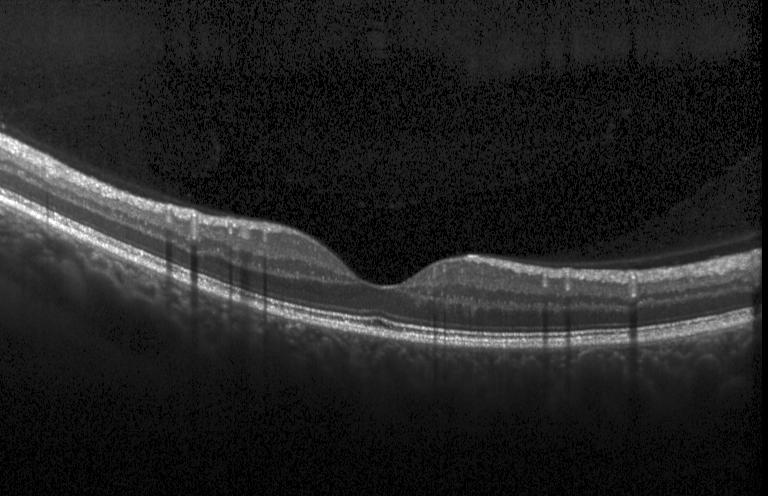
The scan shows no evidence of CNV, DME, or drusen.